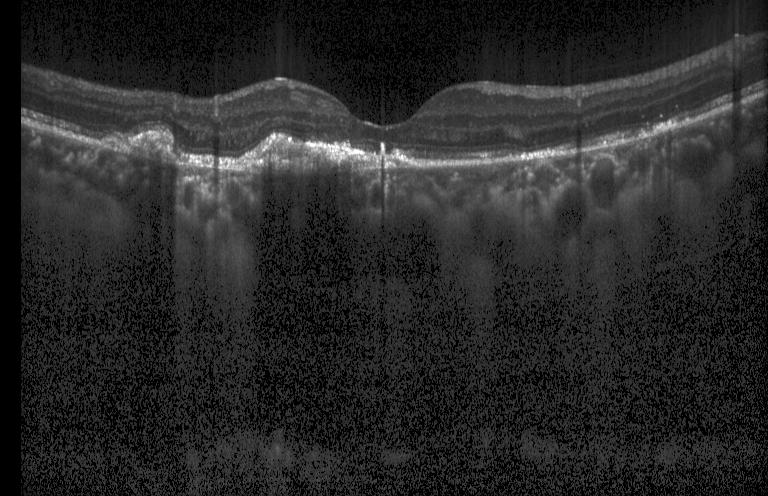

OCT line scan.
Assessment: a choroidal neovascular membrane.